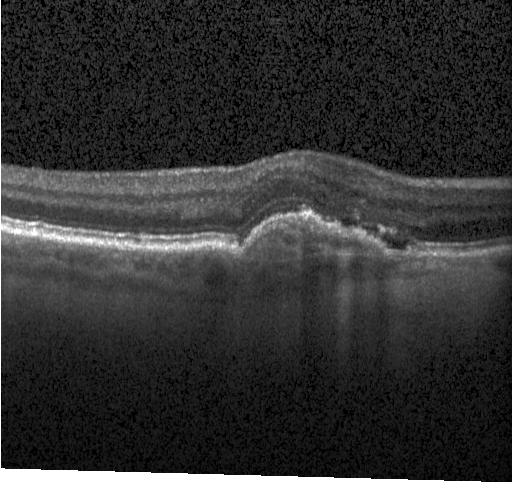
Finding: choroidal neovascularization.